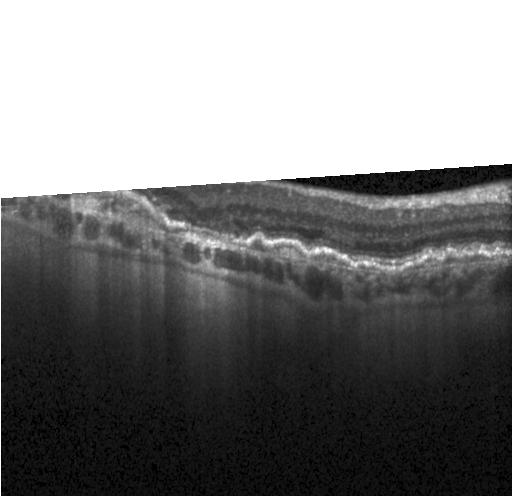

Spectral-domain OCT. Optical coherence tomography B-scan.
Impression: choroidal neovascularization (CNV).